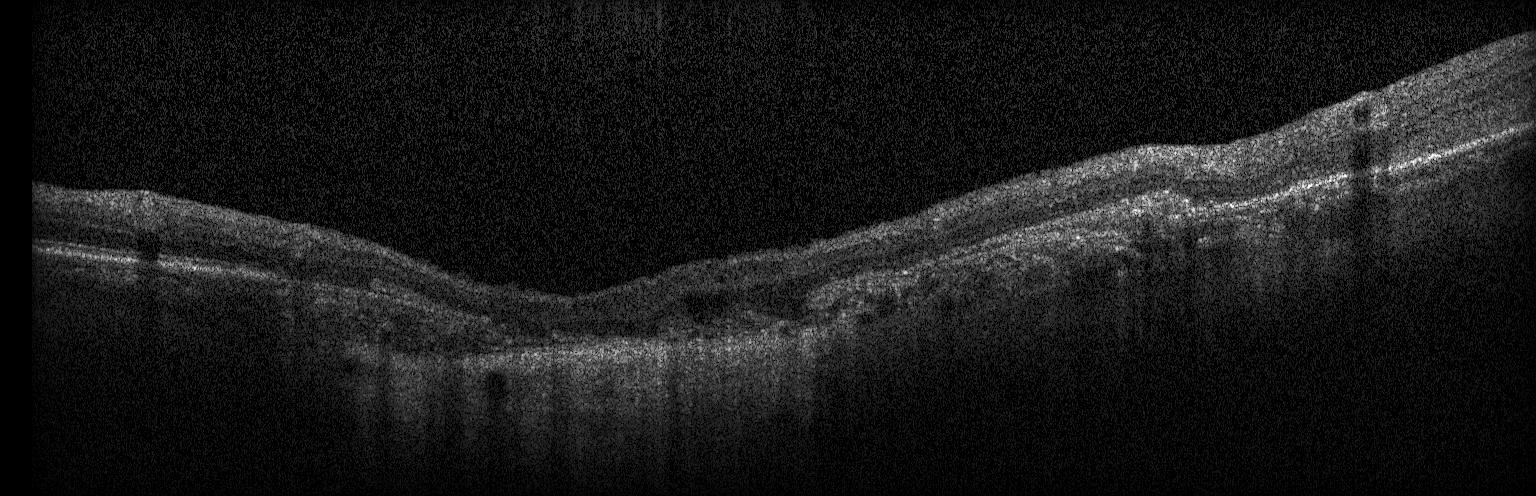 Diagnosis: a choroidal neovascular membrane.